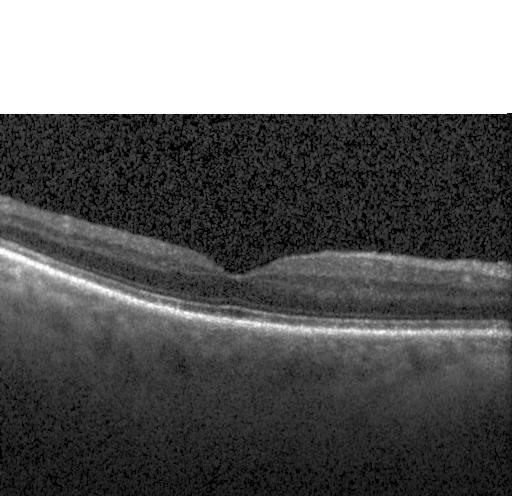

OCT line scan — Impression: no choroidal neovascularization, diabetic macular edema, or drusen.